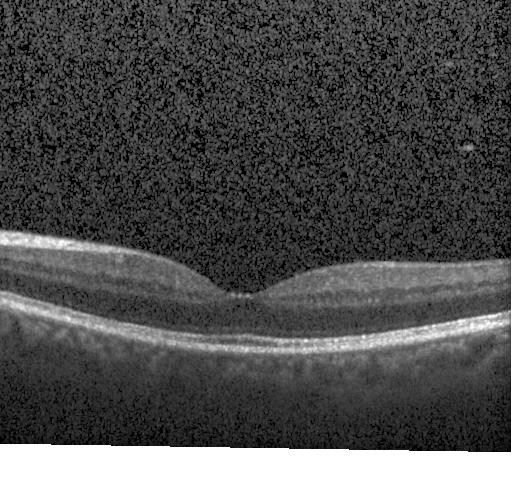
Diagnosis: neither choroidal neovascularization, diabetic macular edema, nor drusen.